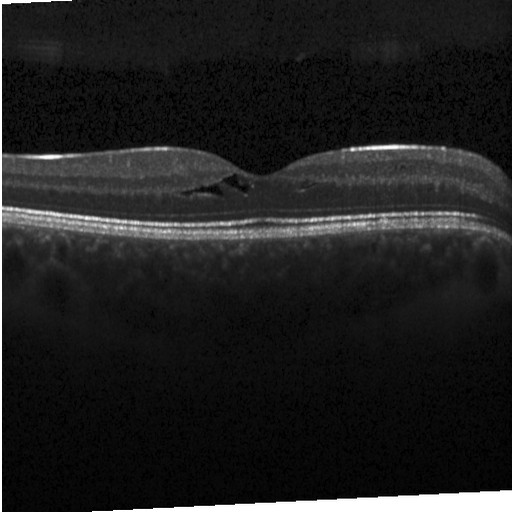
Diabetic macular edema (DME).